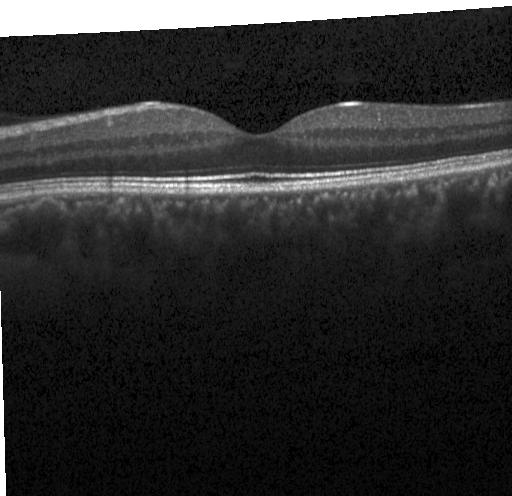

OCT B-scan, macular scan, acquired on a Heidelberg Spectralis
Finding: no CNV, DME, or drusen.